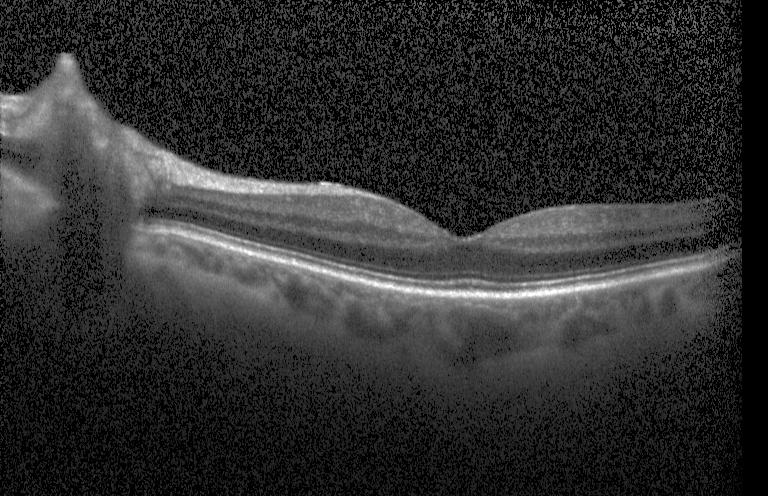

Assessment: no evidence of choroidal neovascularization, diabetic macular edema, or drusen.